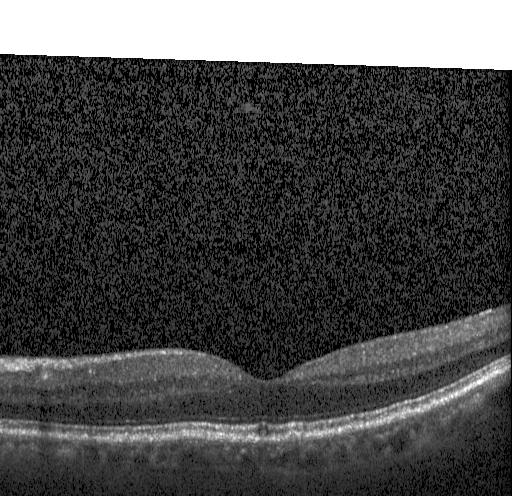

Diagnosis: no choroidal neovascularization, no diabetic macular edema, and no drusen.